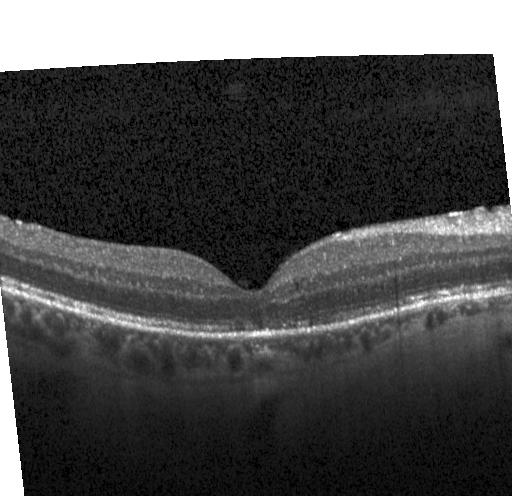 Optical coherence tomography B-scan, acquired on a Heidelberg Spectralis, spectral-domain optical coherence tomography, horizontal scan through the fovea.
Macular OCT: no evidence of CNV, DME, or drusen.